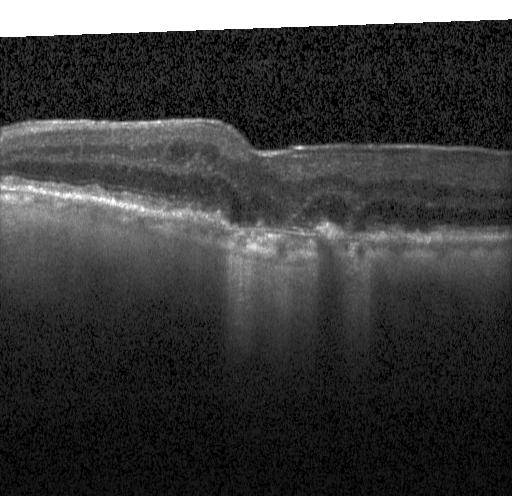 The scan shows a choroidal neovascular membrane.